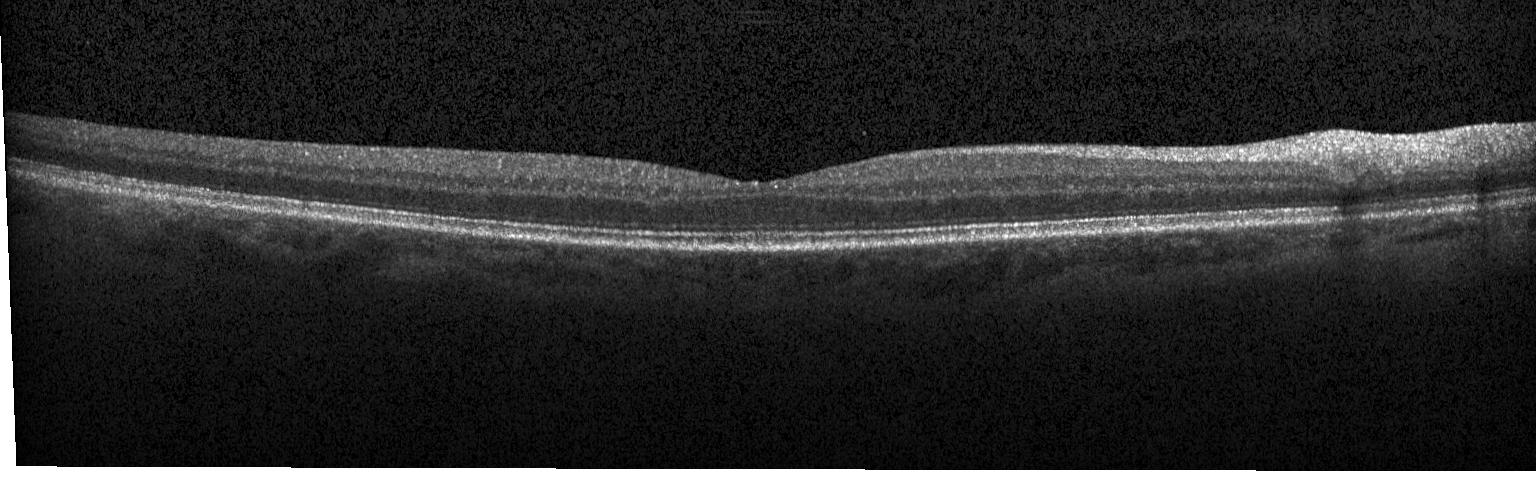

Diagnosis: no choroidal neovascularization, diabetic macular edema, or drusen.